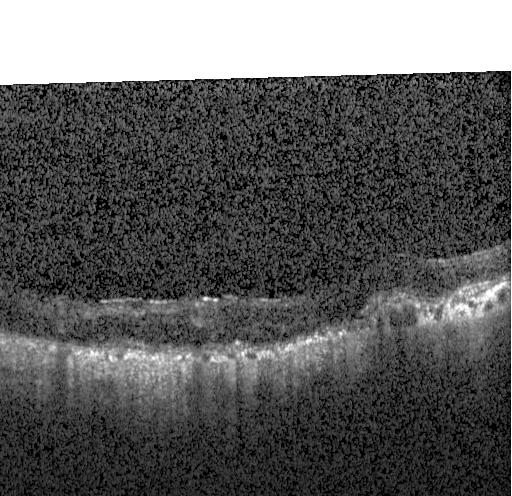
Finding: a choroidal neovascular membrane.